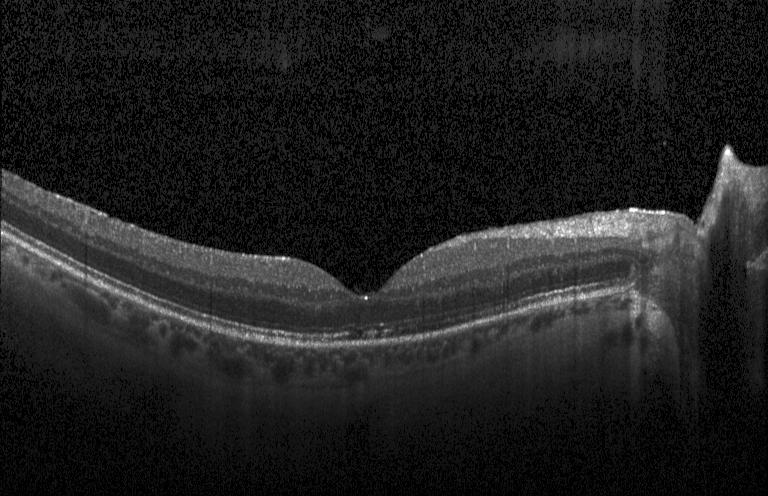 Spectral-domain OCT B-scan: neither CNV, DME, nor drusen.